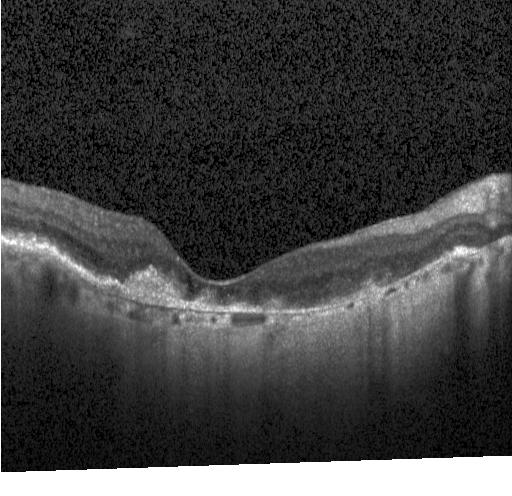

Retinal OCT cross-section showing choroidal neovascularization.